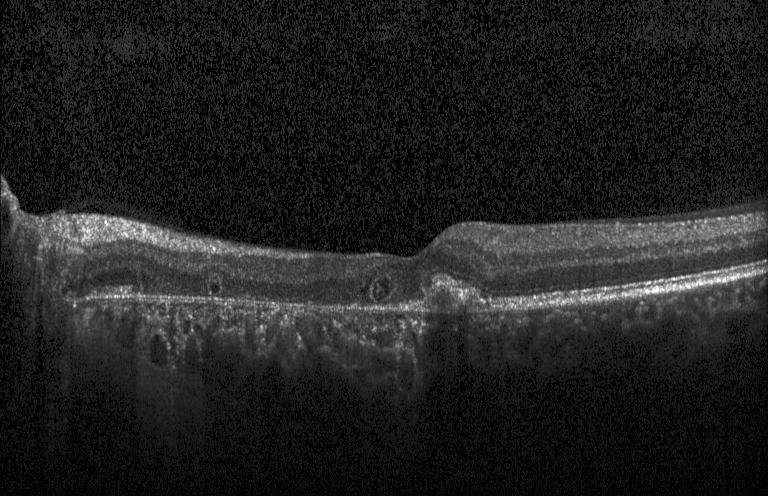
OCT B-scan, horizontal scan through the fovea. The scan shows choroidal neovascularization.